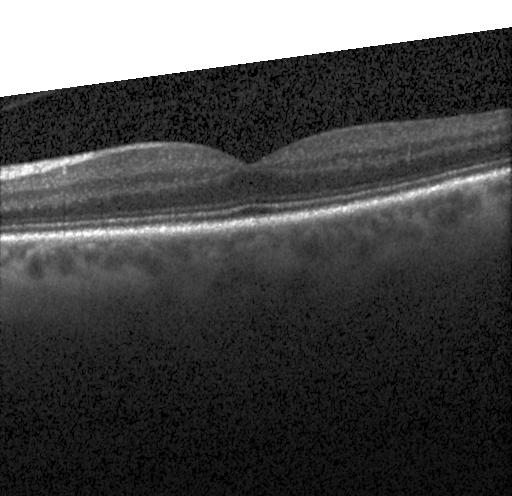
Diagnosis: no choroidal neovascularization, no diabetic macular edema, and no drusen.